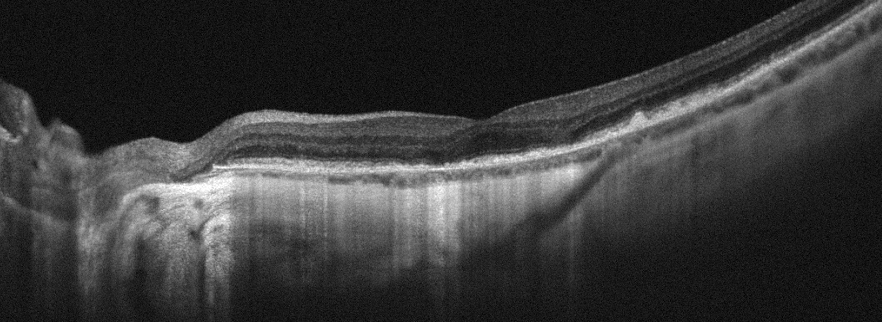
Oculus sinister. Optical coherence tomography B-scan — Impression: AMD.